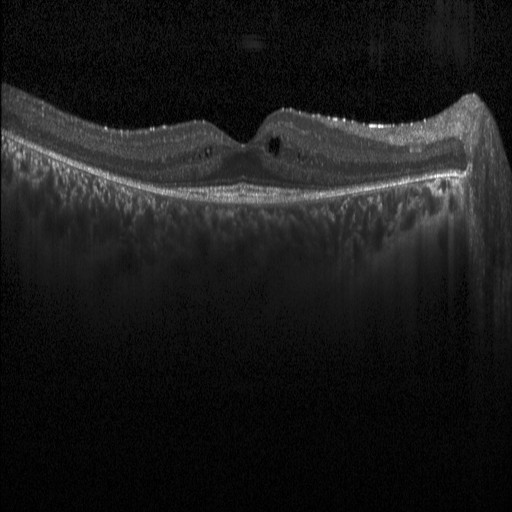
OCT finding: DME.